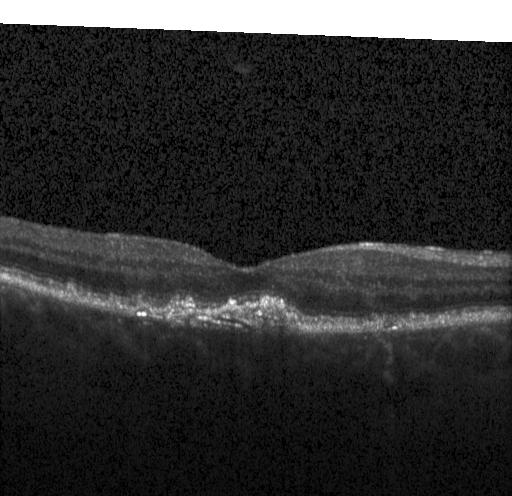
Retinal OCT cross-section showing choroidal neovascularization (CNV).